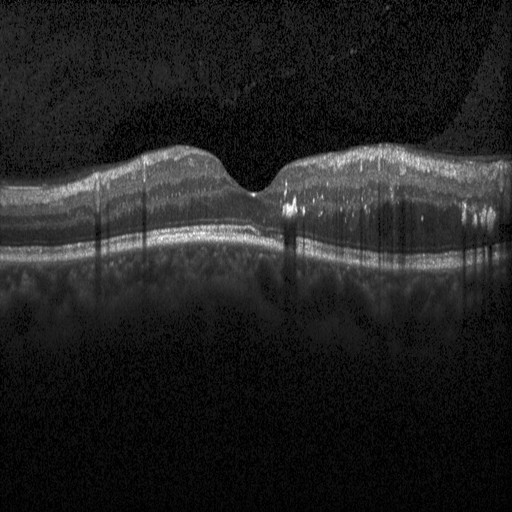
Heidelberg Spectralis; centered on the fovea; spectral-domain OCT; retinal OCT B-scan
This B-scan demonstrates diabetic macular edema.